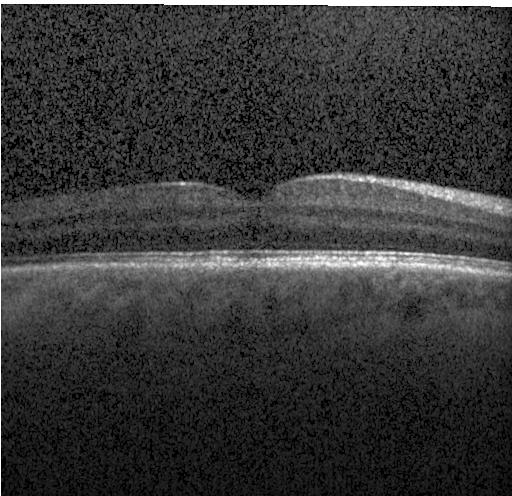

The scan shows neither CNV, DME, nor drusen.